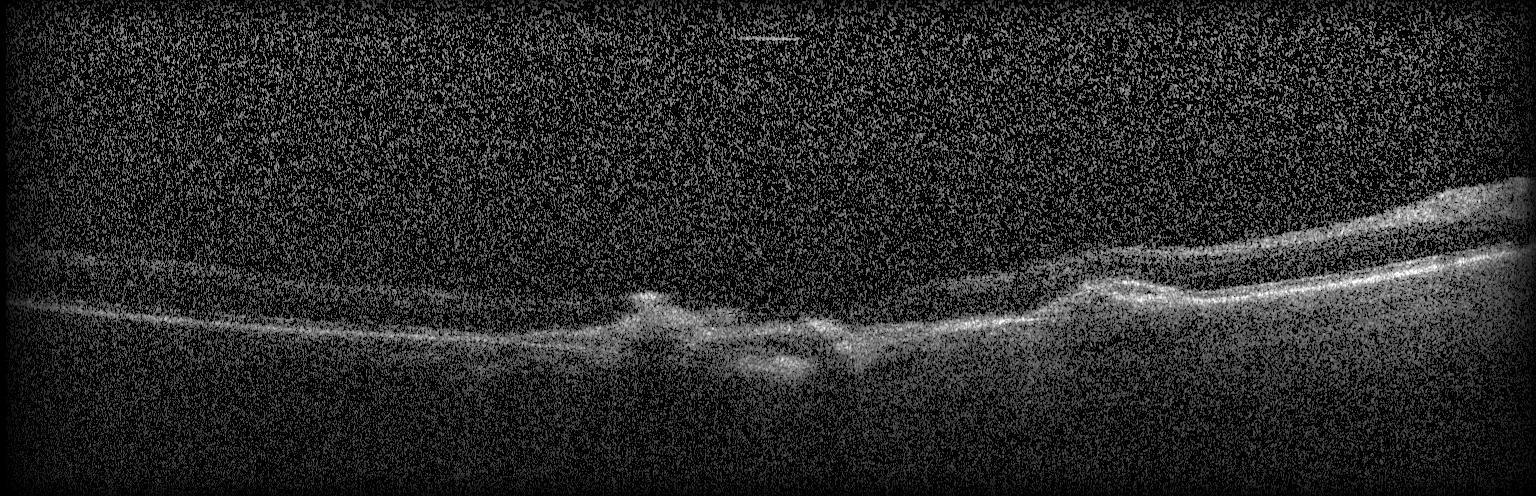 Spectral-domain OCT; OCT line scan; horizontal scan through the fovea. Finding: a choroidal neovascular membrane.